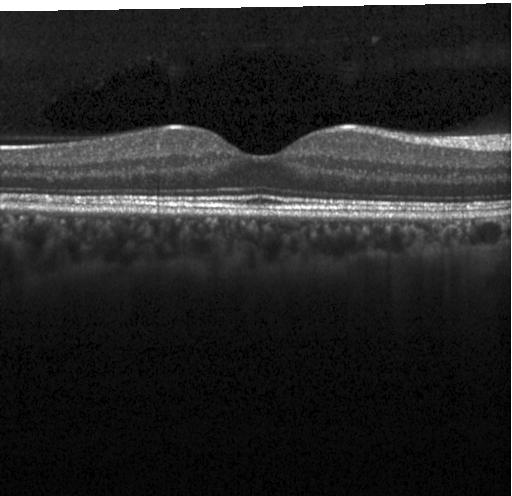
Spectral-domain OCT, Heidelberg Spectralis OCT system, optical coherence tomography B-scan, horizontal scan through the fovea
Finding: no choroidal neovascularization, no diabetic macular edema, and no drusen.